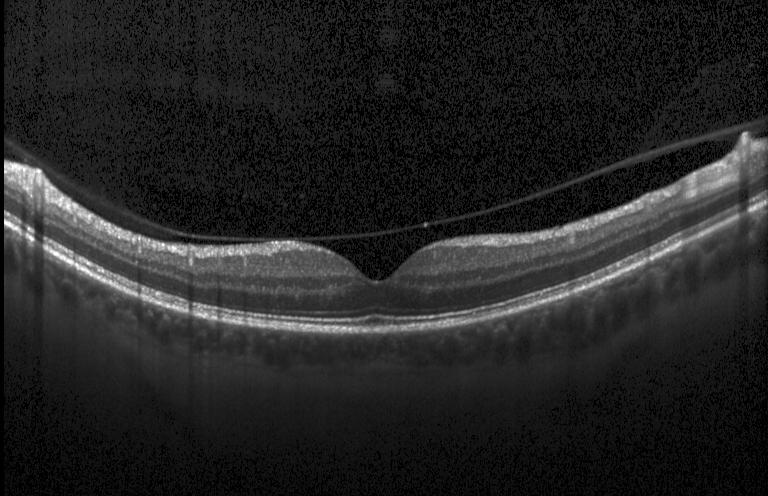

Acquired on a Heidelberg Spectralis. Retinal OCT cross-section. Finding: no evidence of choroidal neovascularization, diabetic macular edema, or drusen.